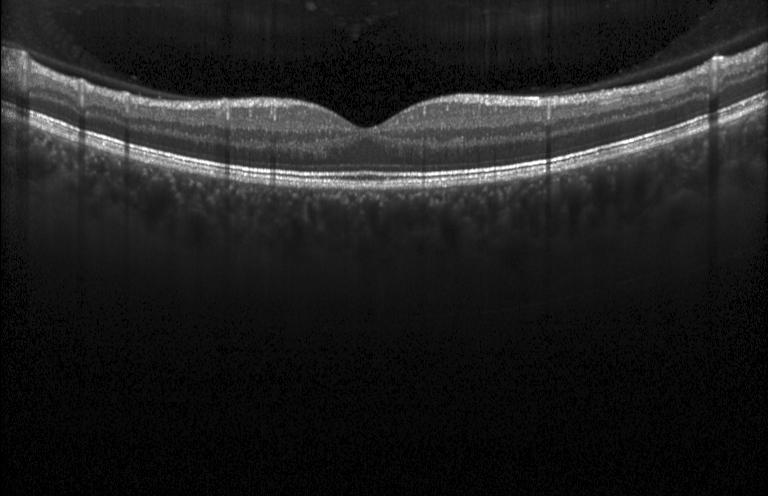
Macular OCT: no evidence of CNV, DME, or drusen.